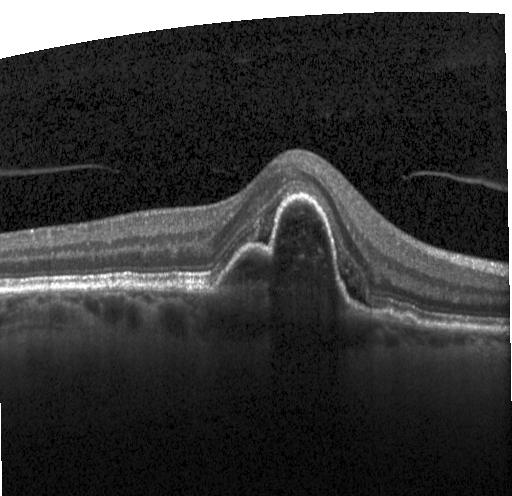

Optical coherence tomography B-scan · Heidelberg Spectralis OCT system · SD-OCT · centered on the fovea — Diagnosis: a choroidal neovascular membrane.